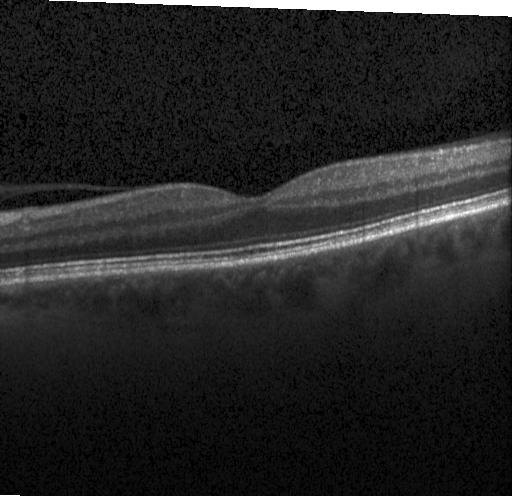 OCT B-scan showing no evidence of choroidal neovascularization, diabetic macular edema, or drusen.